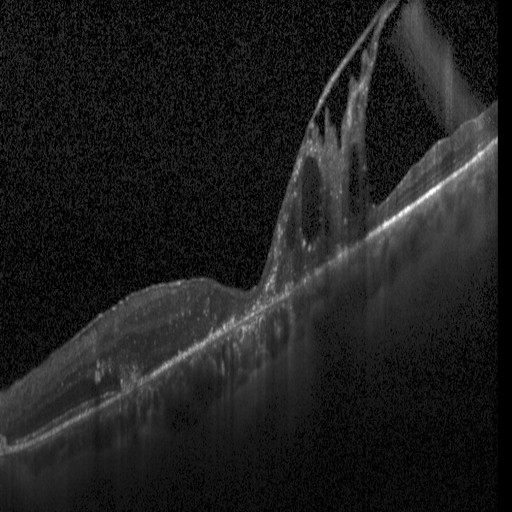
Impression: diabetic macular edema (DME).